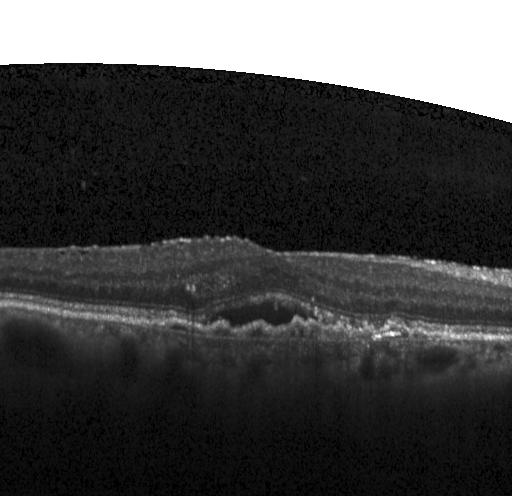 SD-OCT; optical coherence tomography B-scan; macular scan; instrument: Heidelberg Spectralis
Finding: choroidal neovascularization (CNV).